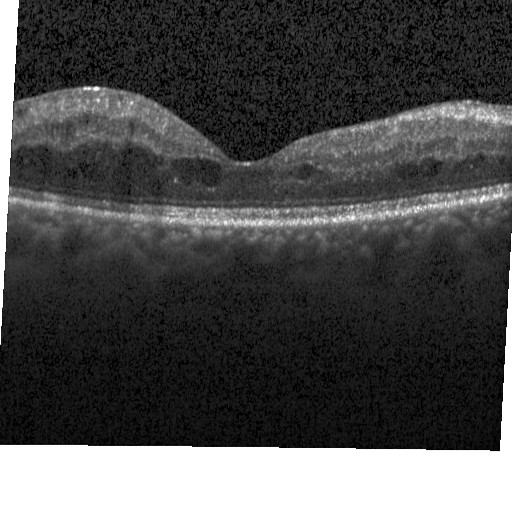

Impression: diabetic macular edema.